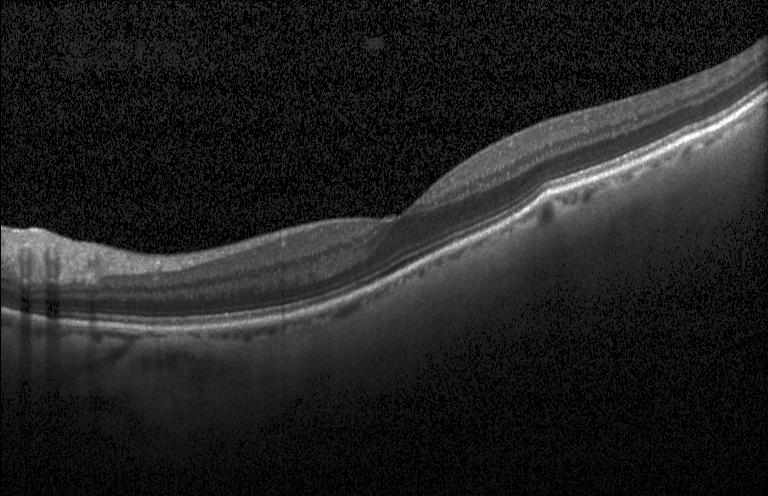 Retinal OCT B-scan.
OCT finding: no choroidal neovascularization, diabetic macular edema, or drusen.